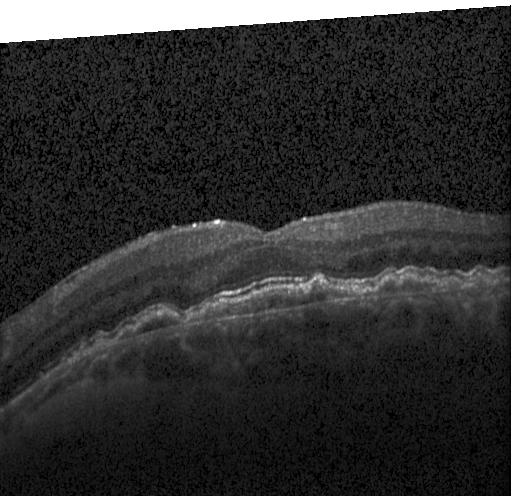
Impression: choroidal neovascularization.